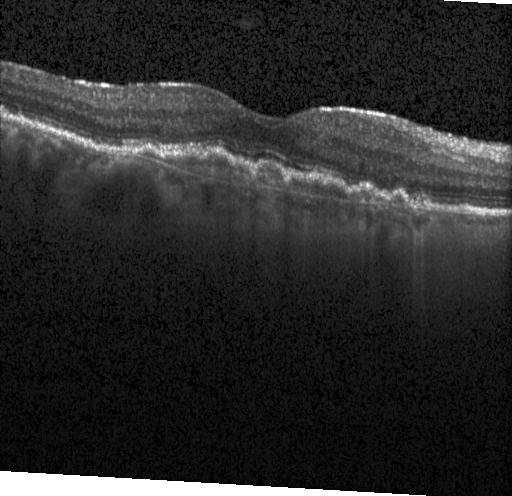

Acquired on a Heidelberg Spectralis · spectral-domain OCT · optical coherence tomography scan · through the macula — Finding: a choroidal neovascular membrane.